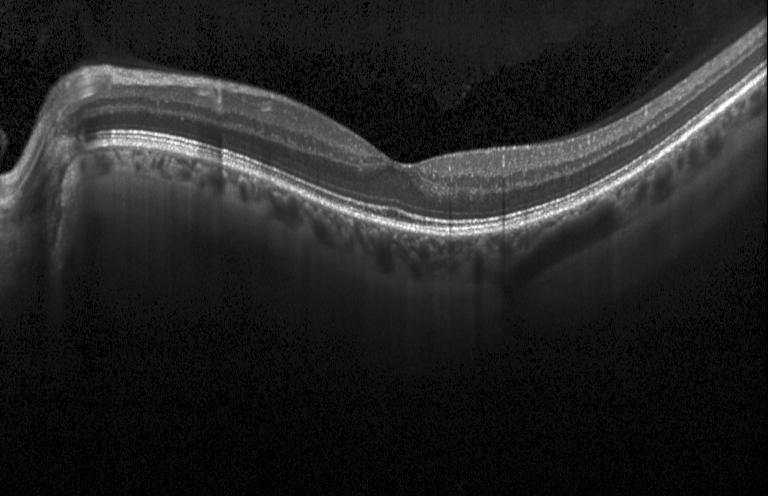
Spectral-domain OCT; fovea-centered; retinal OCT B-scan; Heidelberg Spectralis — Impression: neither choroidal neovascularization, diabetic macular edema, nor drusen.